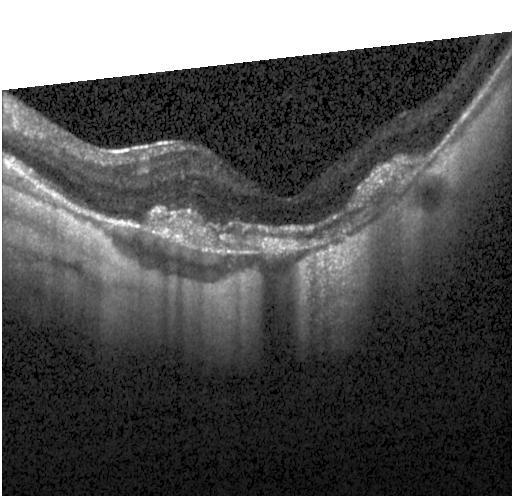

Optical coherence tomography scan, spectral-domain optical coherence tomography, Heidelberg Spectralis OCT system, through the macula
Diagnosis: choroidal neovascularization (CNV).